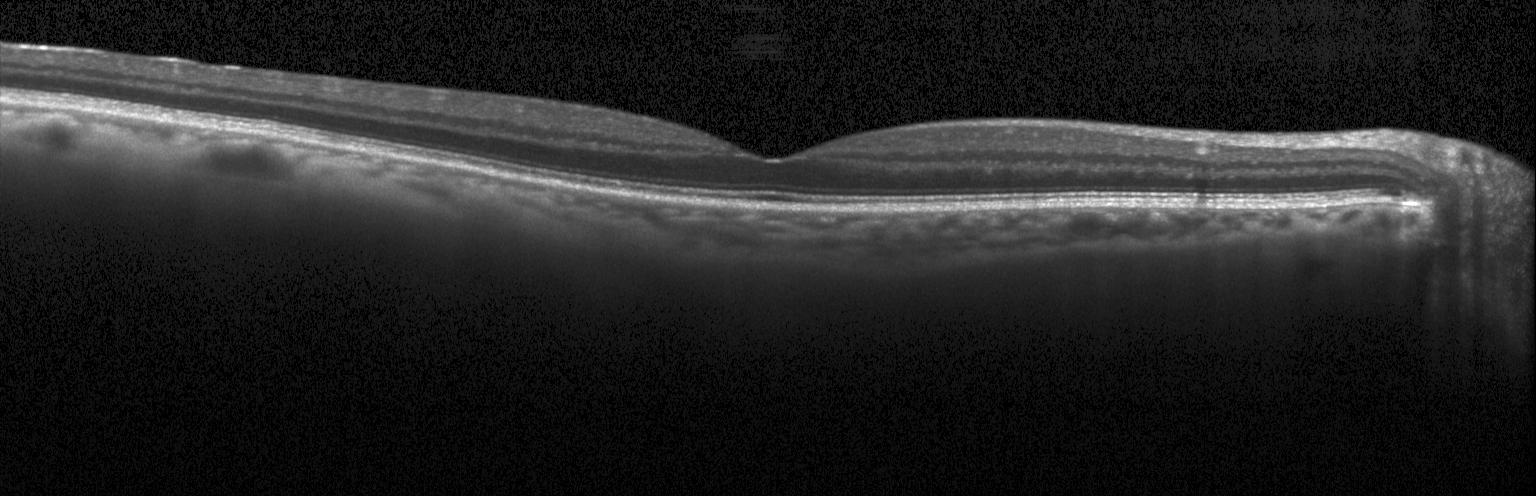

Heidelberg Spectralis; fovea-centered; spectral-domain OCT; optical coherence tomography B-scan
This B-scan demonstrates no choroidal neovascularization, no diabetic macular edema, and no drusen.